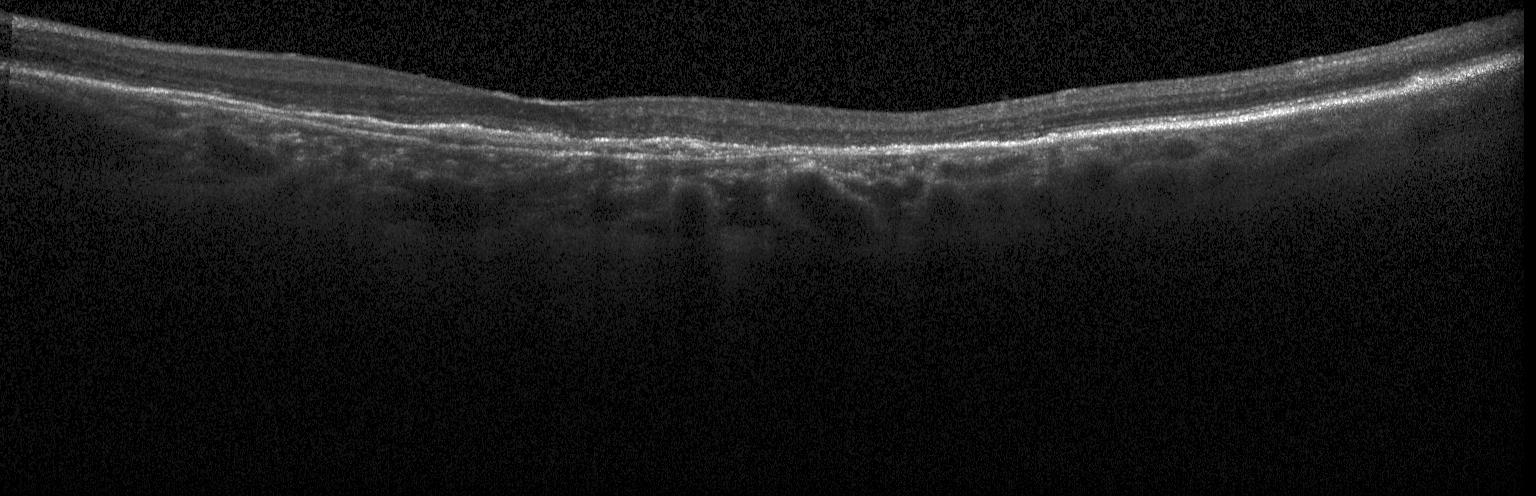
Assessment: a choroidal neovascular membrane.